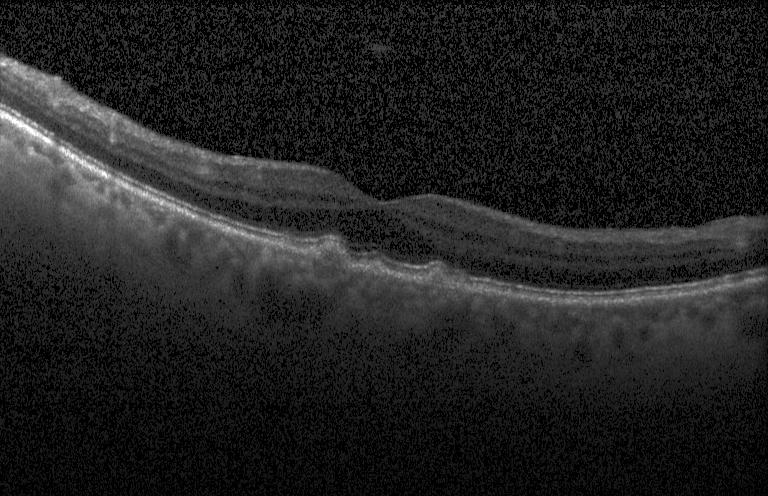 Assessment: drusen.